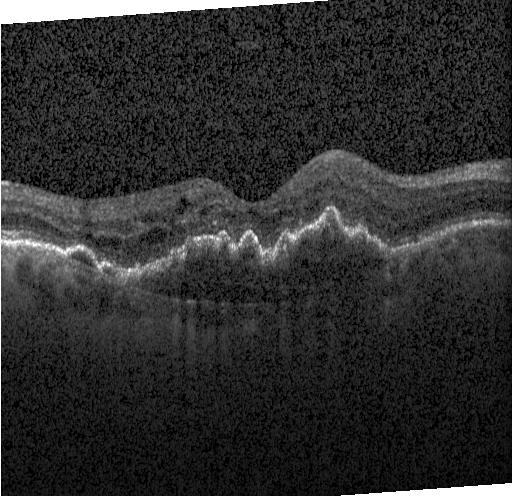

Diagnosis: choroidal neovascularization (CNV).